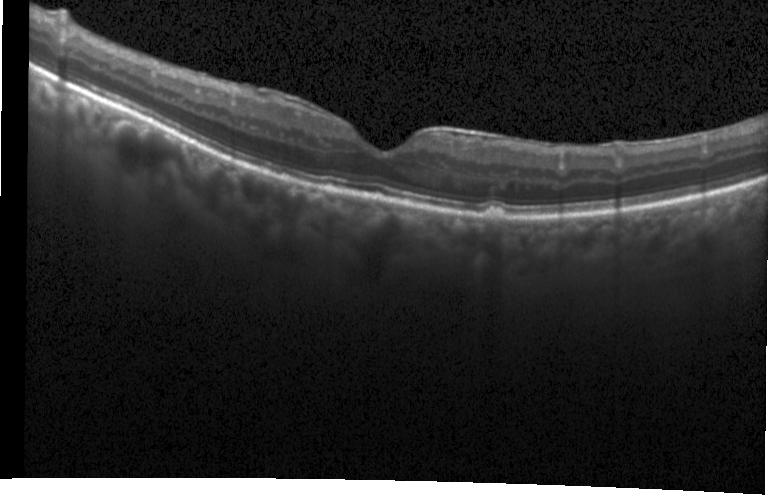 Spectral-domain optical coherence tomography; acquired on a Heidelberg Spectralis; retinal OCT B-scan; macular scan. The scan shows multiple drusen.